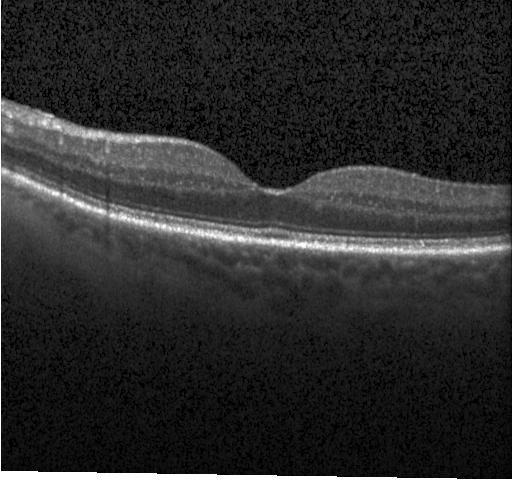
OCT line scan, Heidelberg Spectralis OCT system, SD-OCT.
The scan shows no CNV, no DME, and no drusen.